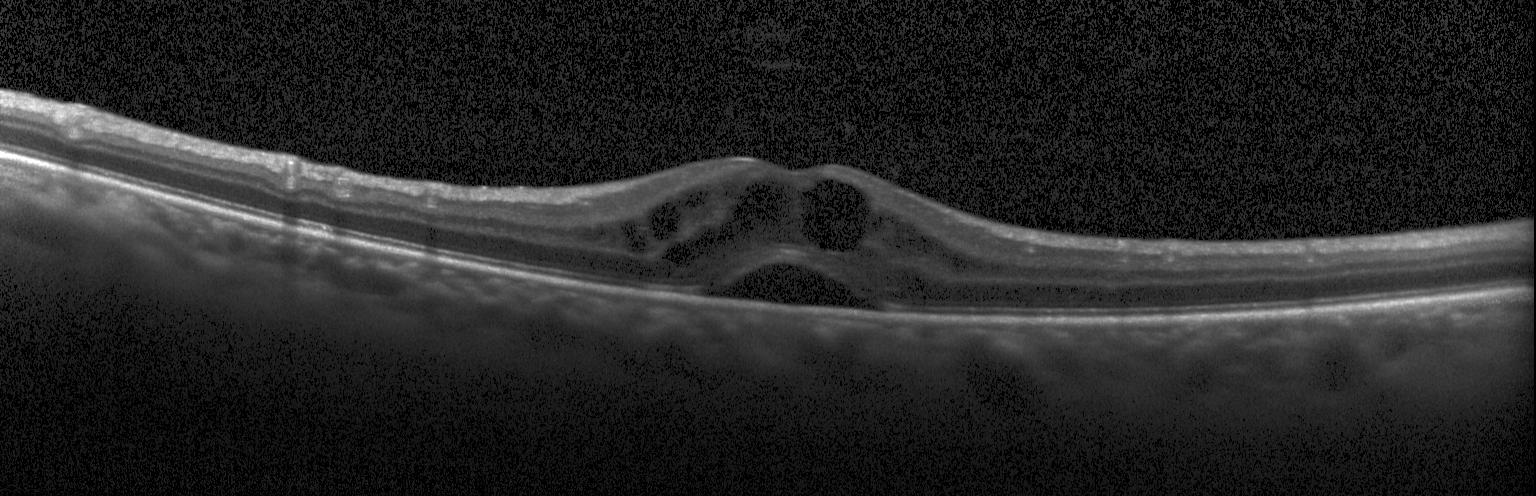 SD-OCT · fovea-centered · optical coherence tomography B-scan.
Dx: diabetic macular edema (DME).